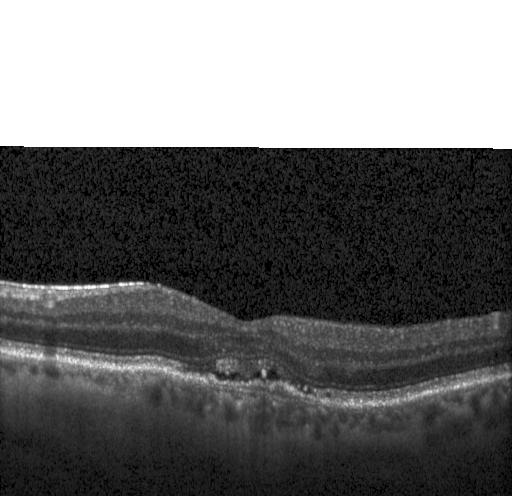 Fovea-centered; spectral-domain optical coherence tomography; acquired on a Heidelberg Spectralis; OCT line scan.
Impression: a choroidal neovascular membrane.